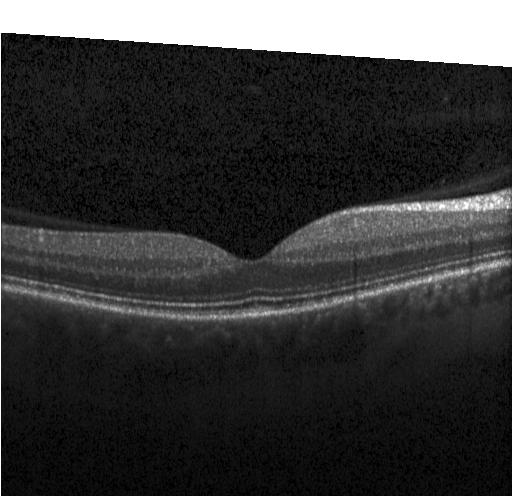

Retinal OCT cross-section showing neither CNV, DME, nor drusen.